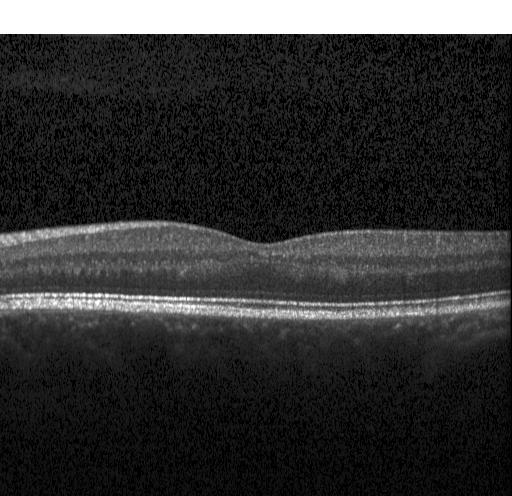 OCT B-scan. Centered on the fovea. Spectral-domain optical coherence tomography
Neither choroidal neovascularization, diabetic macular edema, nor drusen.